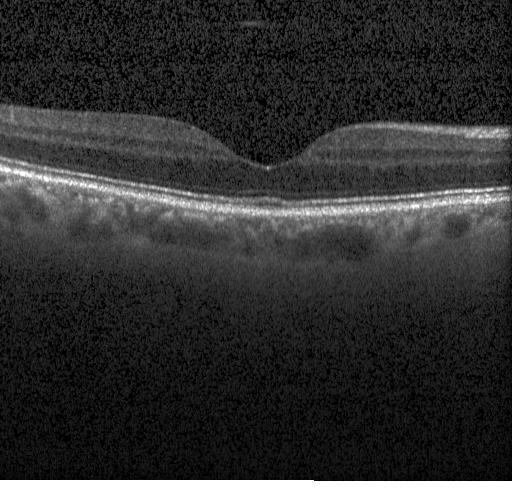

OCT B-scan showing no choroidal neovascularization, diabetic macular edema, or drusen.